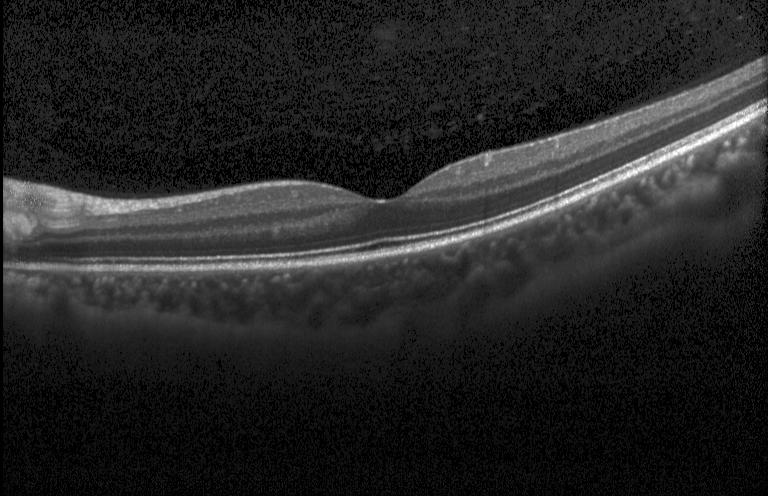

Fovea-centered, optical coherence tomography scan, SD-OCT, Heidelberg Spectralis OCT system. Finding: no choroidal neovascularization, no diabetic macular edema, and no drusen.